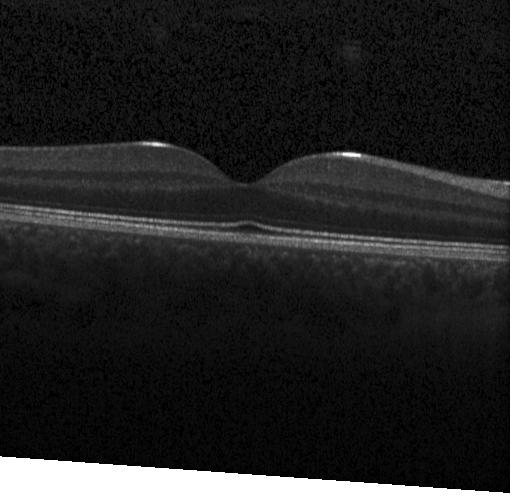
OCT B-scan · through the macula · Heidelberg Spectralis OCT system.
Assessment: neither CNV, DME, nor drusen.